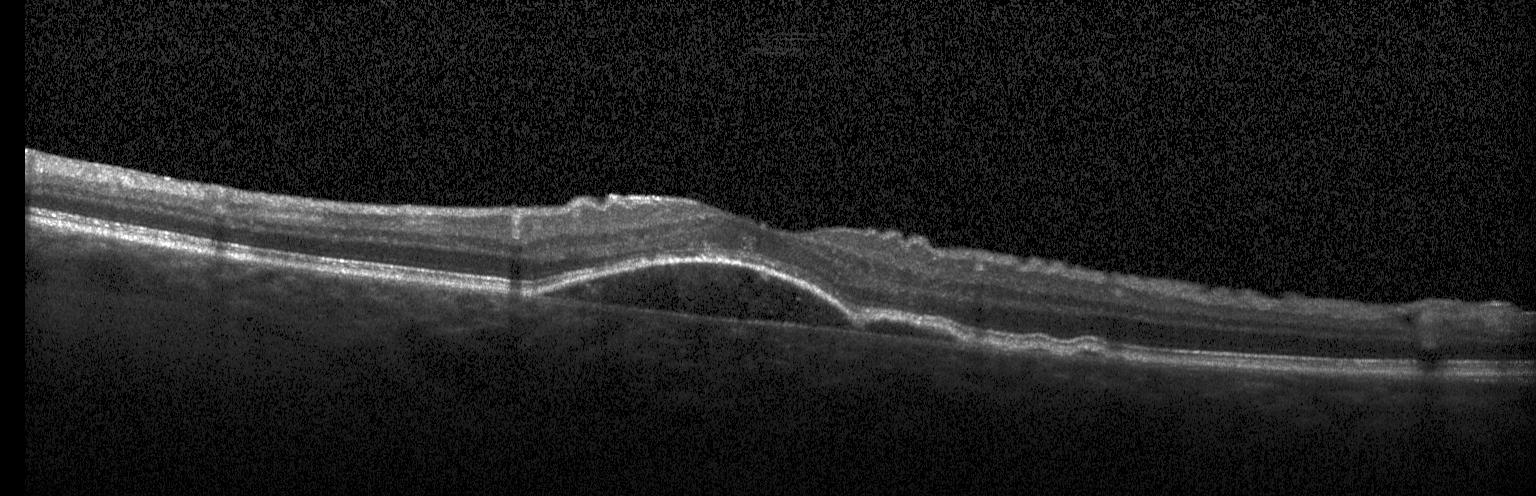 Diagnosis: a choroidal neovascular membrane.